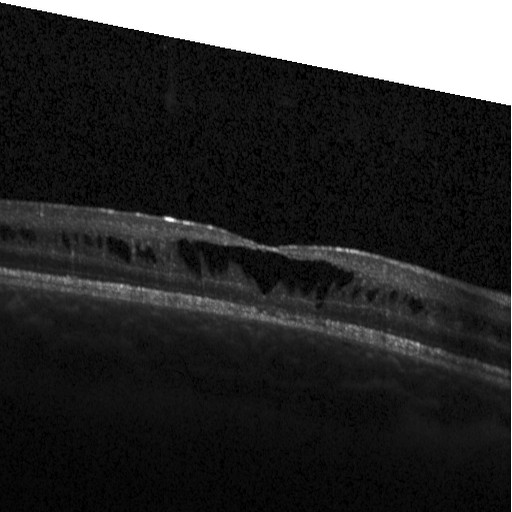

DME.